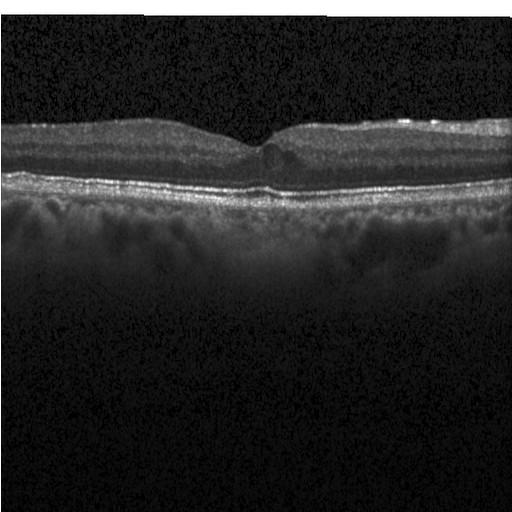

Impression: diabetic macular edema.